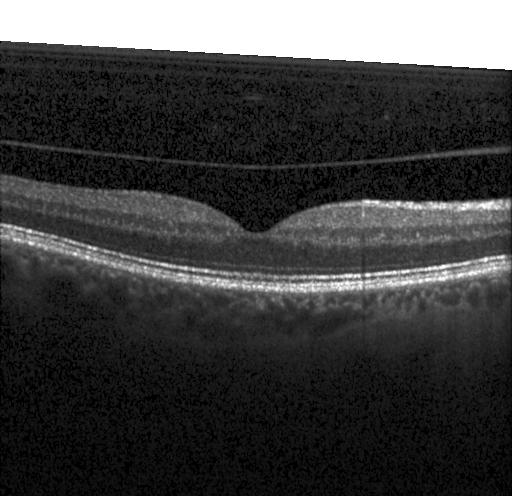 Acquired on a Heidelberg Spectralis, SD-OCT, retinal OCT cross-section.
Neither choroidal neovascularization, diabetic macular edema, nor drusen.